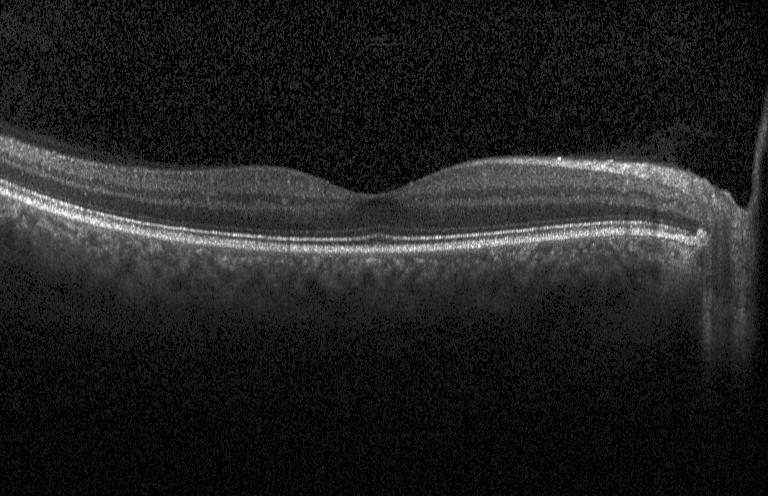

The scan shows no choroidal neovascularization, diabetic macular edema, or drusen.